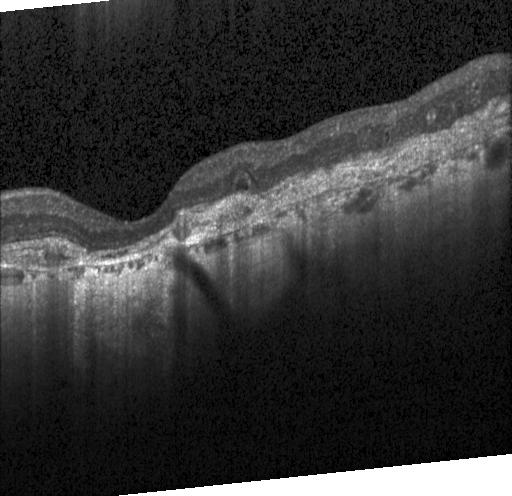

OCT line scan.
This B-scan demonstrates a choroidal neovascular membrane.